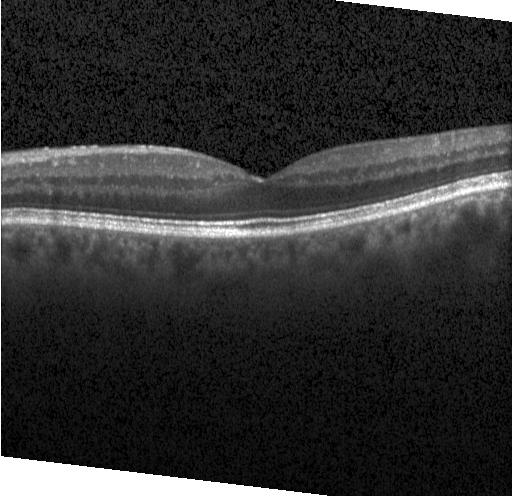
Optical coherence tomography scan. Heidelberg Spectralis OCT system. Spectral-domain OCT — Finding: no choroidal neovascularization, diabetic macular edema, or drusen.